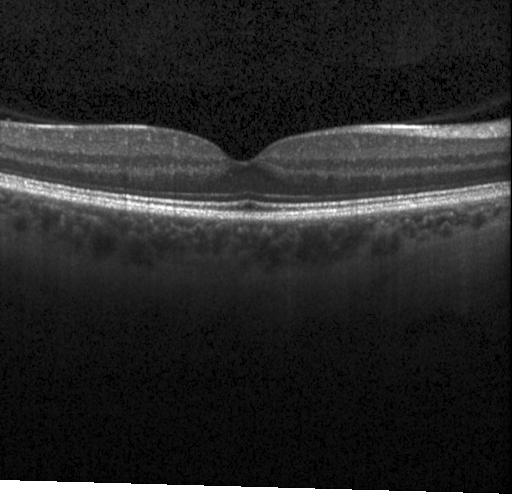
OCT line scan.
Neither CNV, DME, nor drusen.